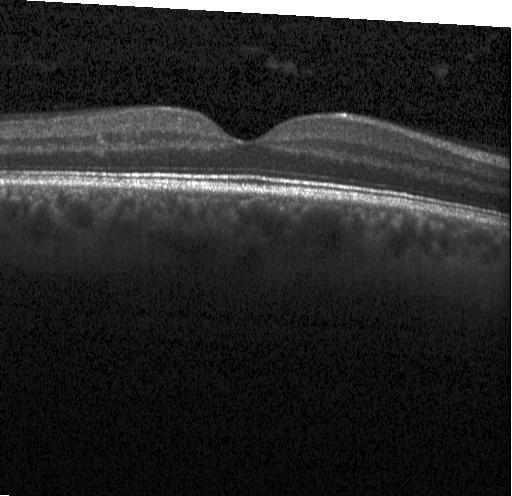
Diagnosis: no choroidal neovascularization, no diabetic macular edema, and no drusen.